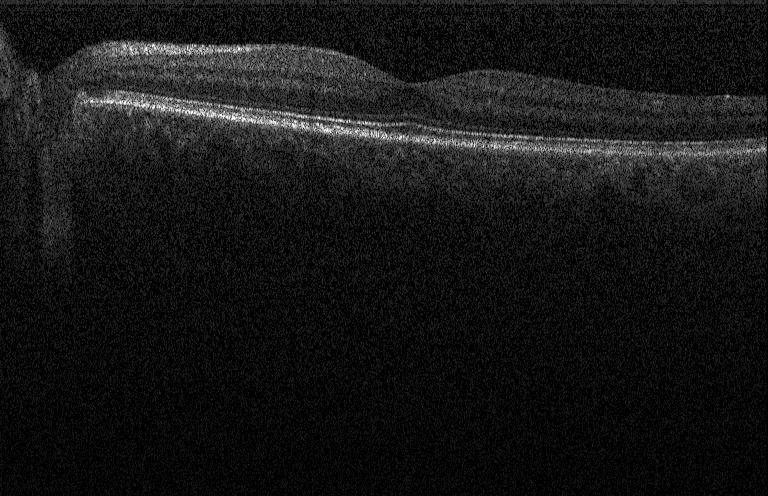 Macular OCT: no evidence of CNV, DME, or drusen.